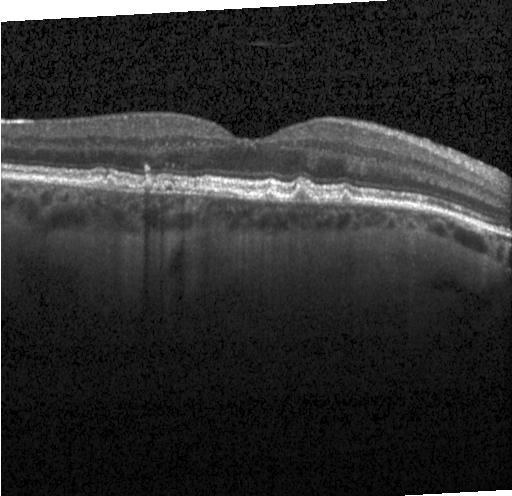

Optical coherence tomography scan. Macular scan. Spectral-domain optical coherence tomography. Impression: multiple drusen.